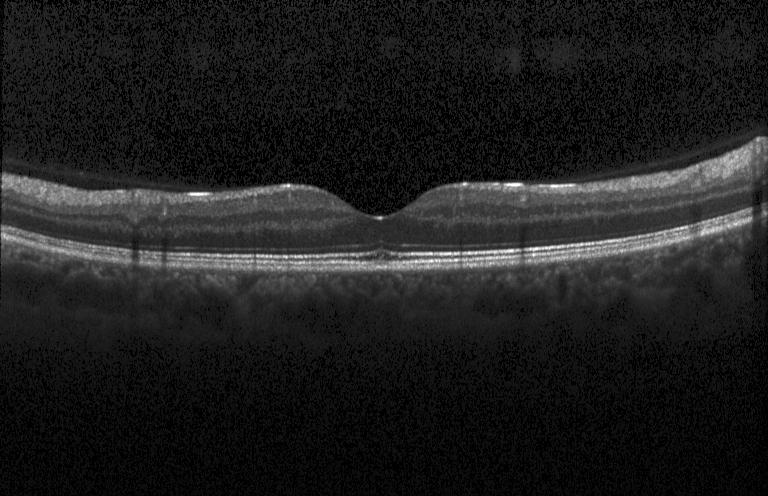 Spectral-domain OCT · centered on the fovea · retinal OCT cross-section — The scan shows no choroidal neovascularization, no diabetic macular edema, and no drusen.